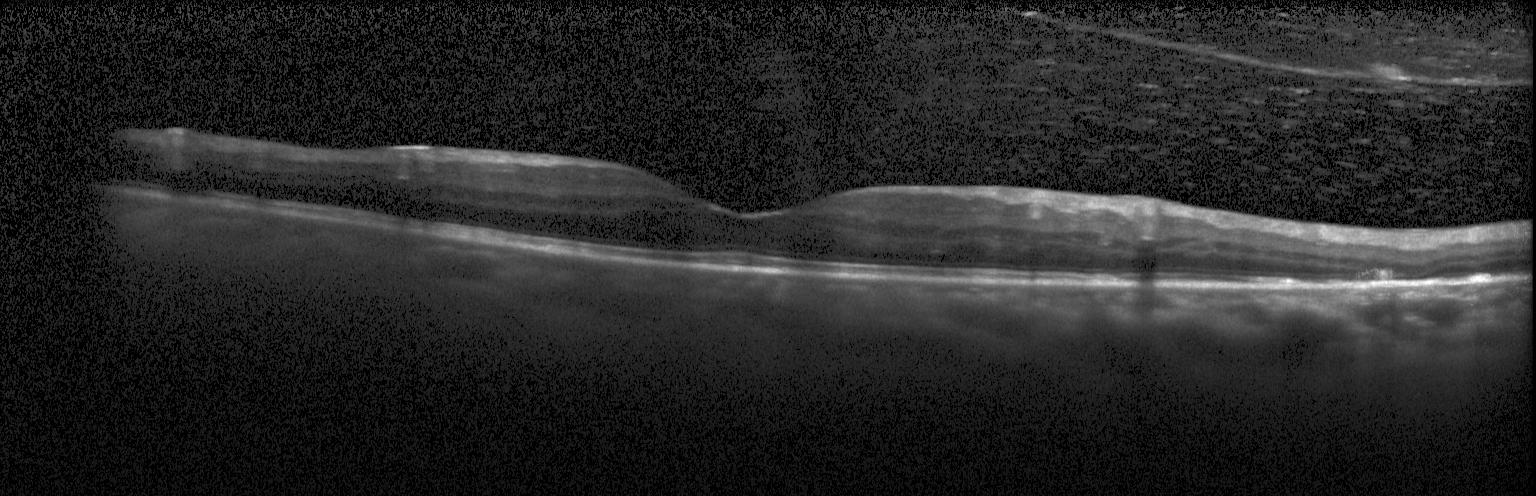

Optical coherence tomography B-scan · acquired on a Heidelberg Spectralis · macular scan
Impression: diabetic macular edema.